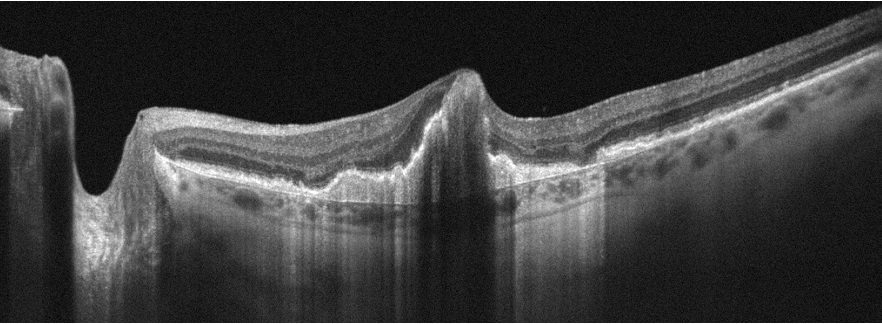
Optical coherence tomography scan
Impression: age-related macular degeneration.